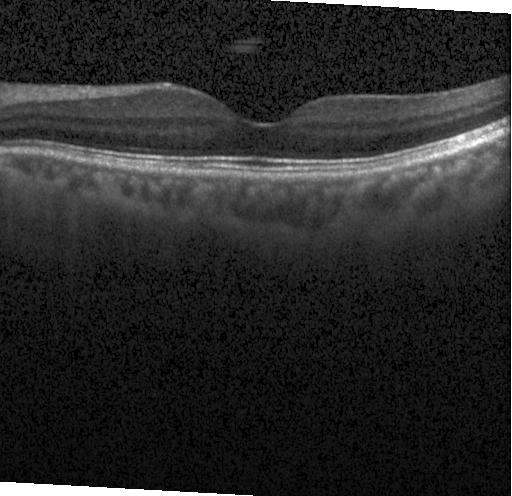 OCT line scan; spectral-domain optical coherence tomography; centered on the fovea; acquired on a Heidelberg Spectralis — Dx: neither choroidal neovascularization, diabetic macular edema, nor drusen.